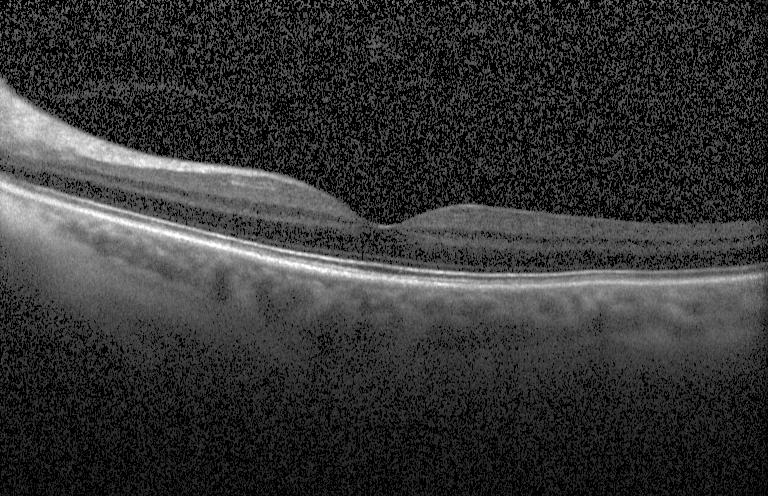
Retinal OCT B-scan · macular scan · Heidelberg Spectralis — Dx: no choroidal neovascularization, no diabetic macular edema, and no drusen.